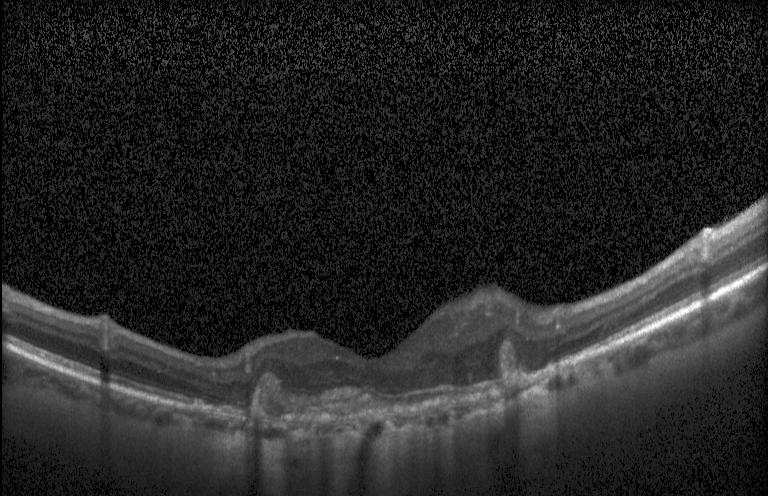
Diagnosis: a choroidal neovascular membrane.